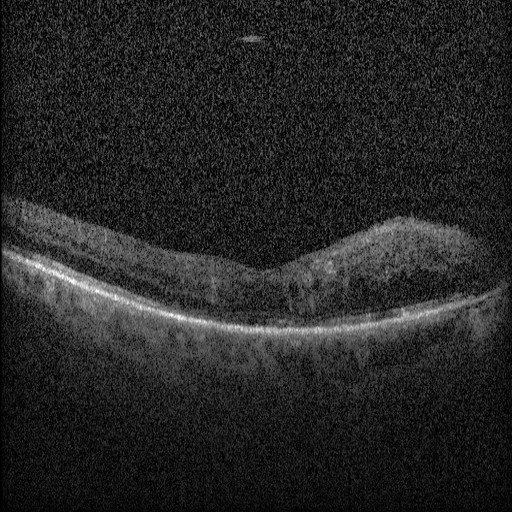

Impression: diabetic macular edema.